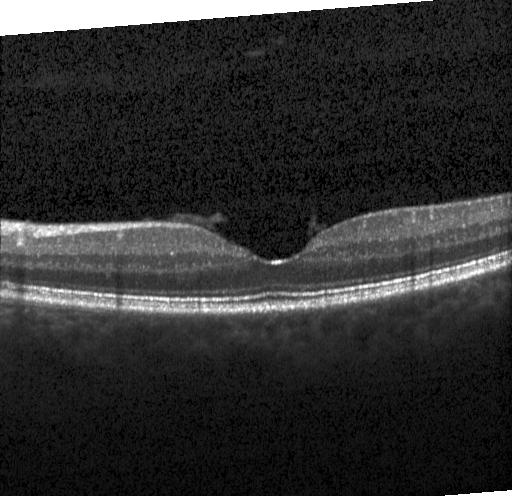

OCT B-scan · acquired on a Heidelberg Spectralis — Dx: no choroidal neovascularization, no diabetic macular edema, and no drusen.